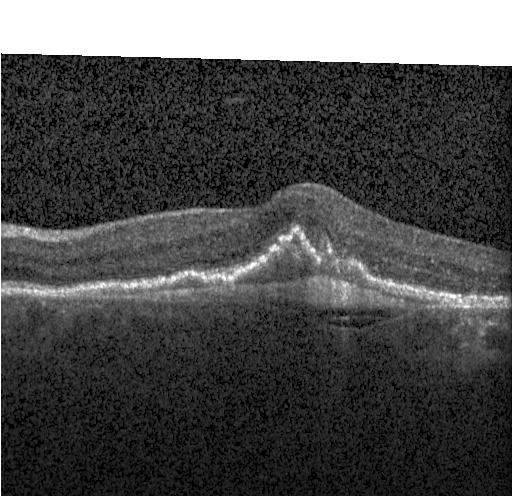

Acquired on a Heidelberg Spectralis, spectral-domain OCT, retinal OCT cross-section, centered on the fovea — OCT finding: a choroidal neovascular membrane.